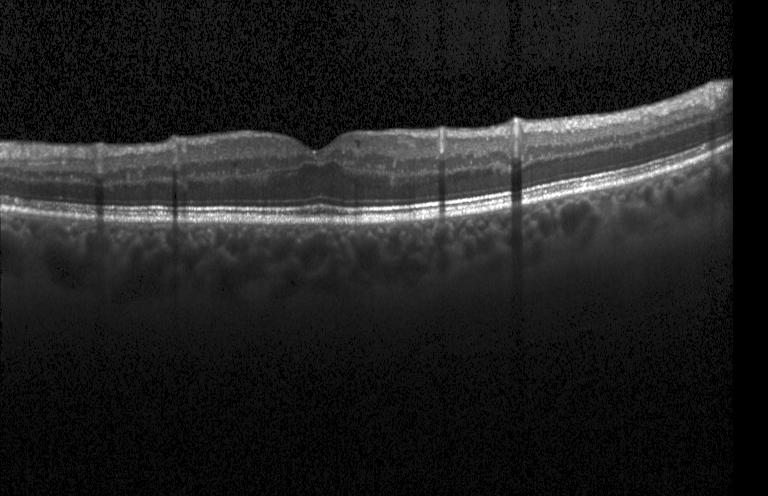

Horizontal scan through the fovea · spectral-domain optical coherence tomography · OCT B-scan · Heidelberg Spectralis OCT system
Diagnosis: no choroidal neovascularization, no diabetic macular edema, and no drusen.